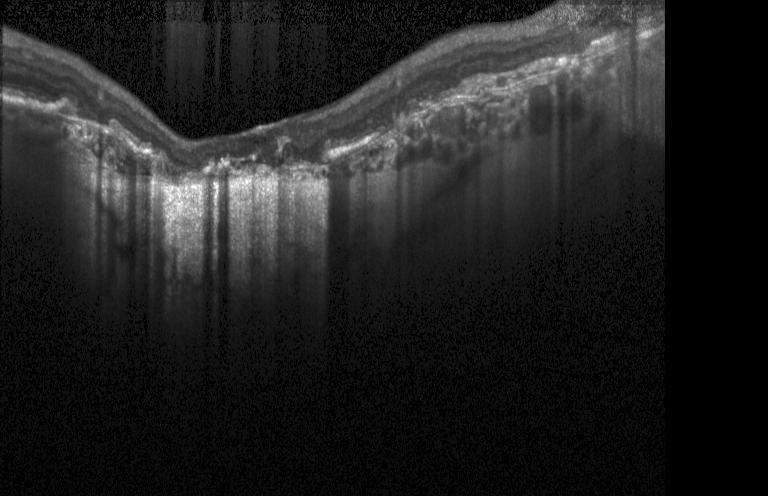
OCT line scan — This B-scan demonstrates a choroidal neovascular membrane.